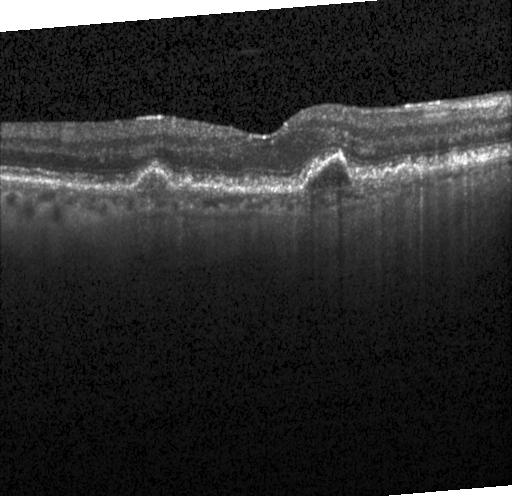

Optical coherence tomography scan. Finding: a choroidal neovascular membrane.